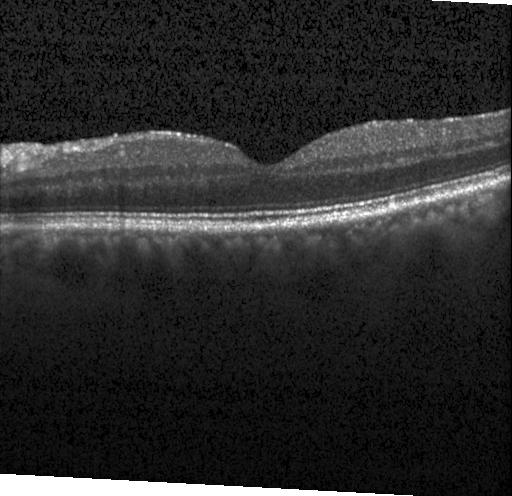 Optical coherence tomography scan; spectral-domain OCT; fovea-centered
Finding: neither choroidal neovascularization, diabetic macular edema, nor drusen.